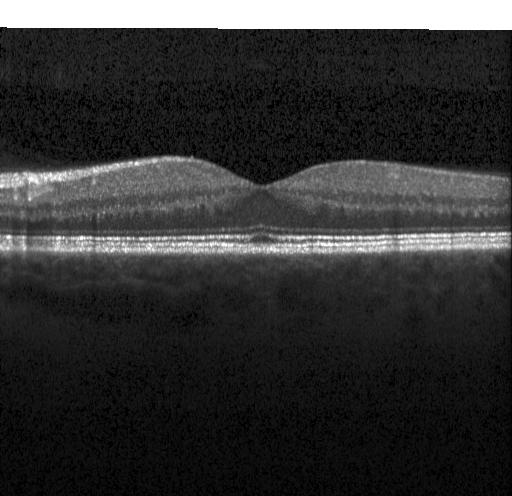
Retinal OCT cross-section showing no choroidal neovascularization, diabetic macular edema, or drusen.